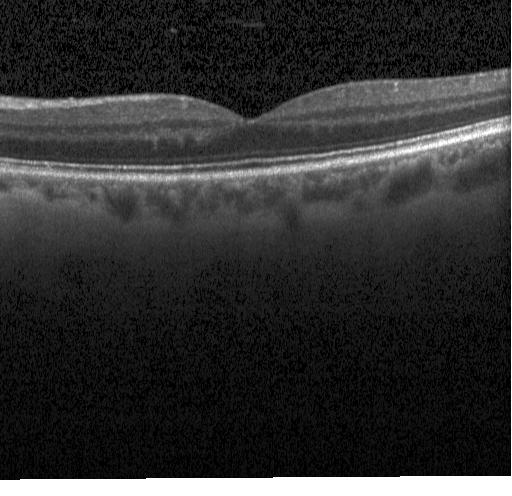

OCT B-scan
Diagnosis: no choroidal neovascularization, no diabetic macular edema, and no drusen.